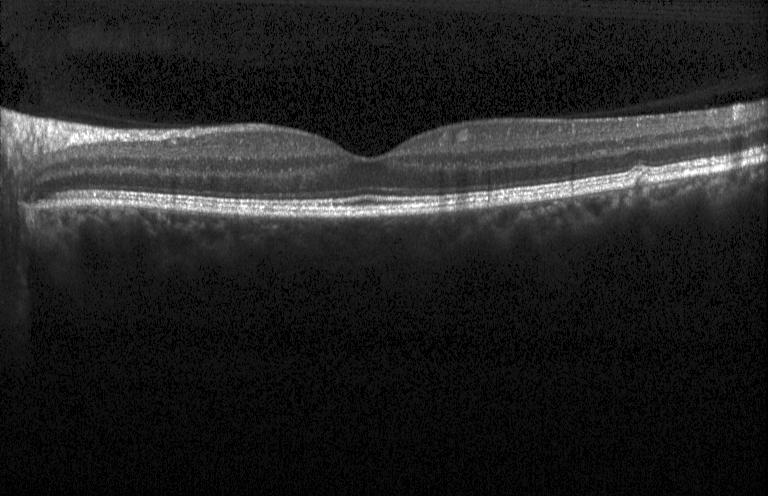 Retinal OCT B-scan. Instrument: Heidelberg Spectralis — Finding: multiple drusen.